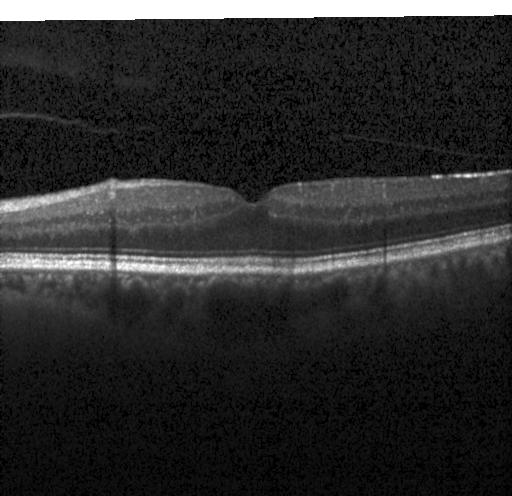 Finding: no choroidal neovascularization, diabetic macular edema, or drusen.